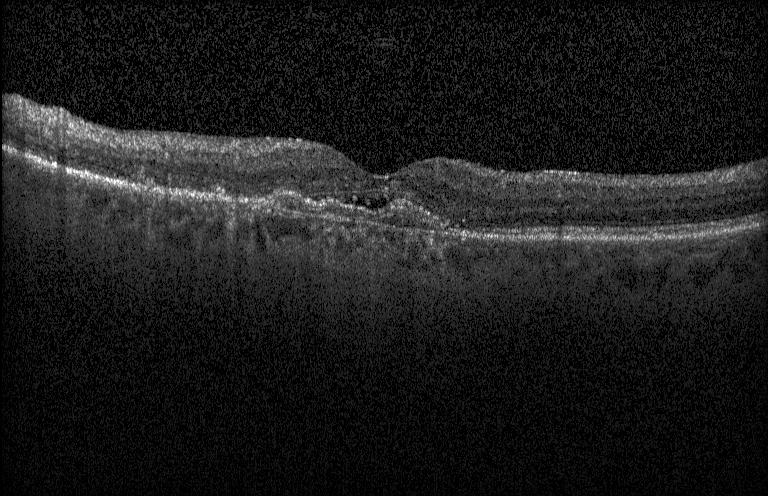
The scan shows CNV.